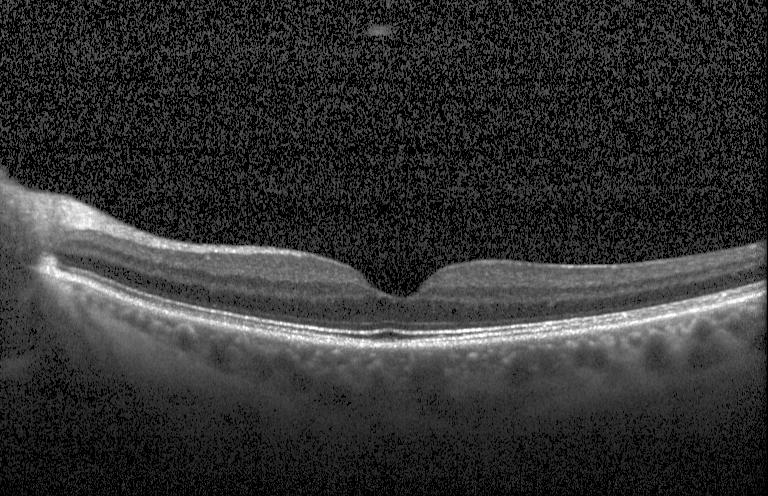

OCT B-scan. Instrument: Heidelberg Spectralis. Impression: no evidence of CNV, DME, or drusen.